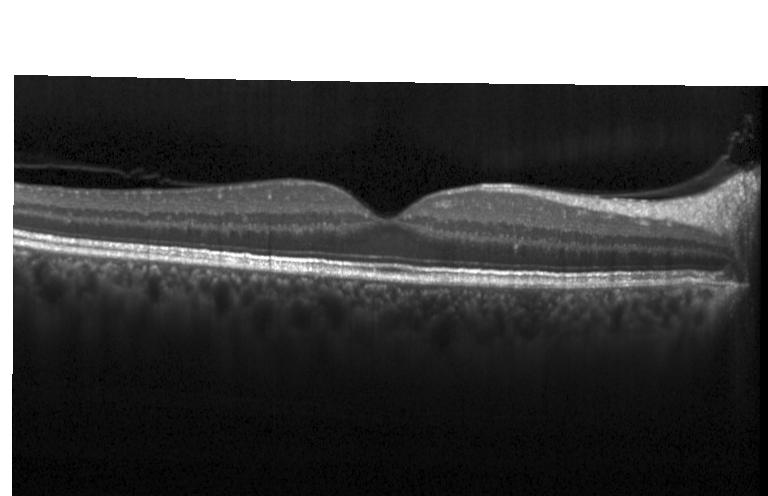
Finding: no choroidal neovascularization, diabetic macular edema, or drusen.